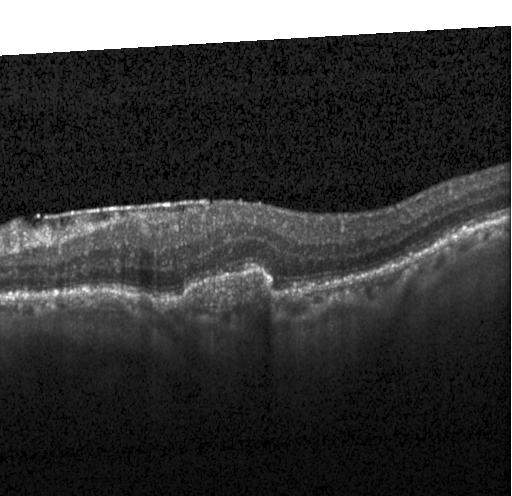
OCT B-scan, Heidelberg Spectralis — Dx: choroidal neovascularization.